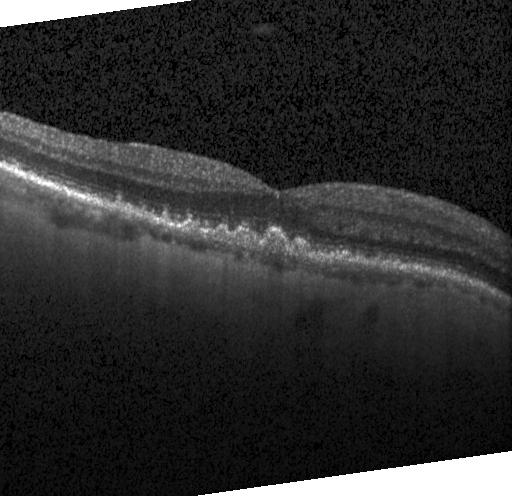

Retinal OCT cross-section. Heidelberg Spectralis OCT system
Finding: sub-RPE drusenoid deposits.